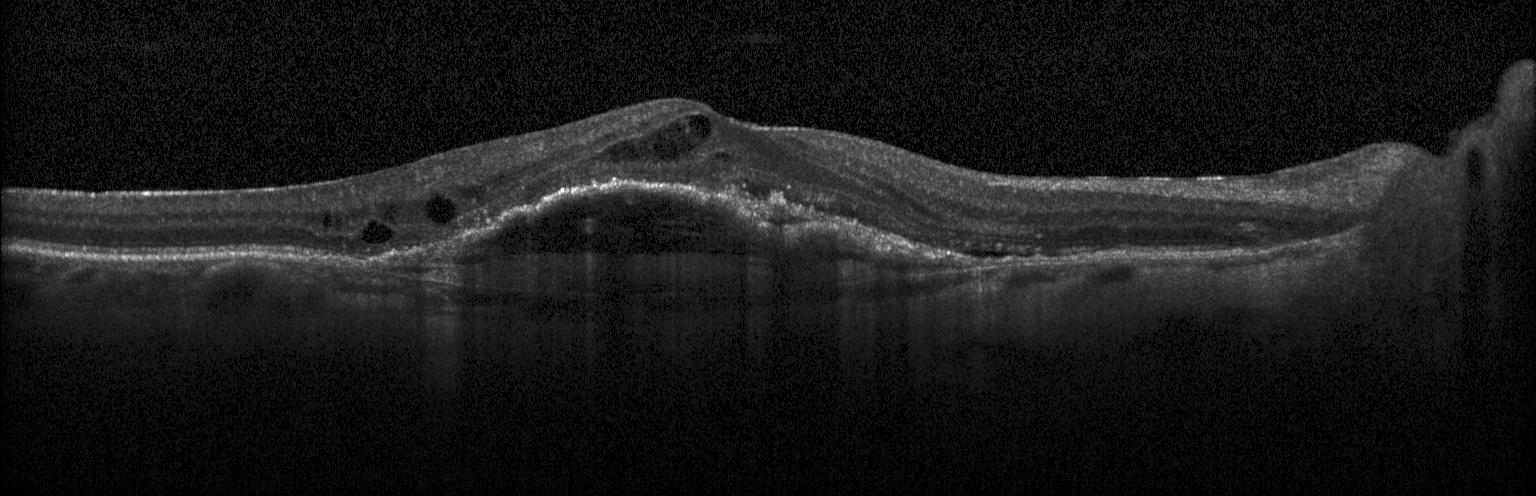

Macular scan, spectral-domain OCT, optical coherence tomography B-scan — Finding: a choroidal neovascular membrane.